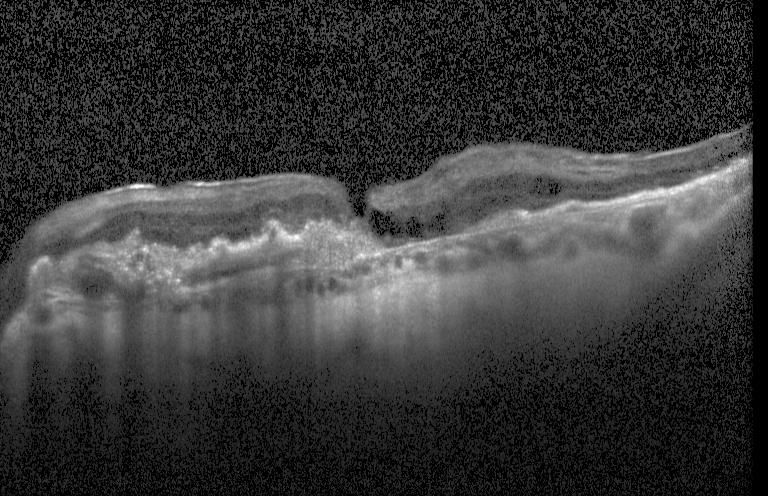

Optical coherence tomography B-scan; instrument: Heidelberg Spectralis; fovea-centered. Impression: a choroidal neovascular membrane.